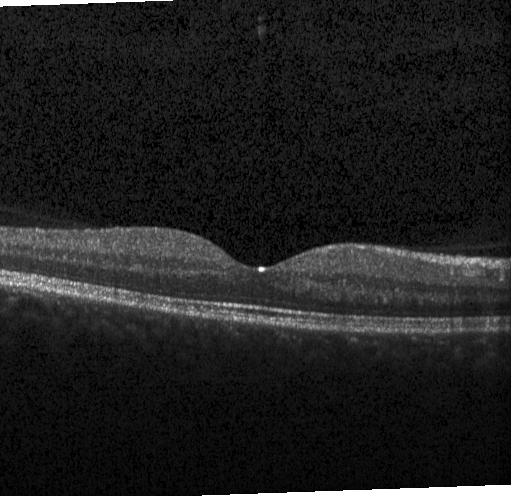

Impression: no choroidal neovascularization, no diabetic macular edema, and no drusen.